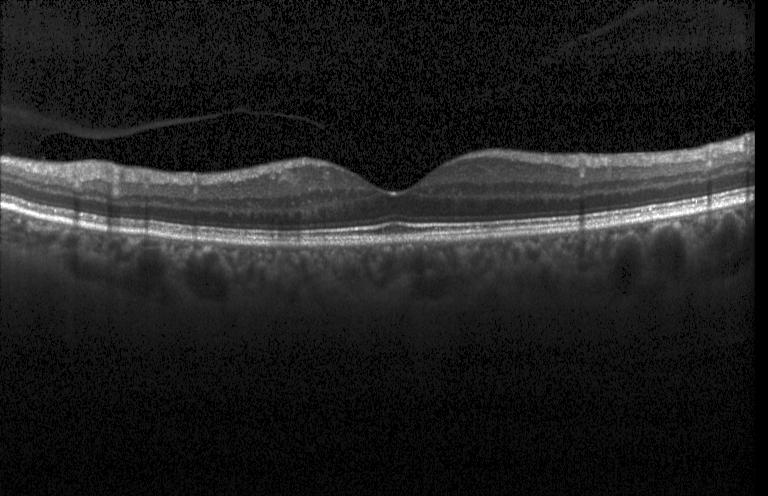
Retinal OCT B-scan, centered on the fovea
No choroidal neovascularization, diabetic macular edema, or drusen.